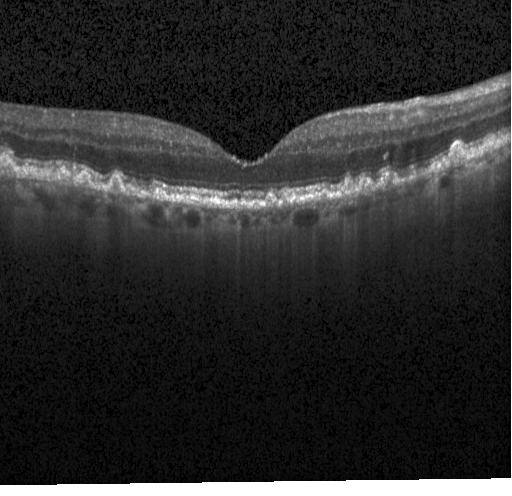 Retinal OCT cross-section — Macular OCT: sub-RPE drusenoid deposits.